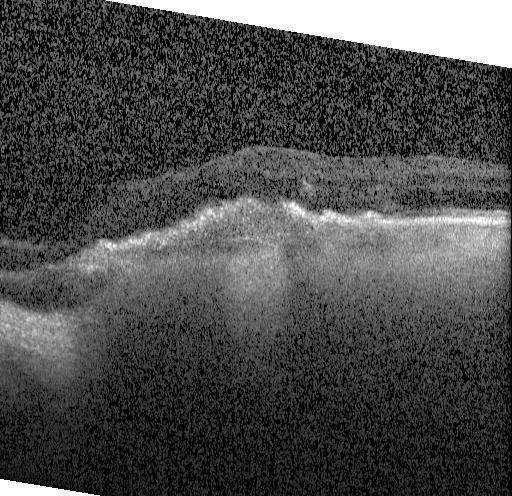 OCT B-scan.
Impression: CNV.